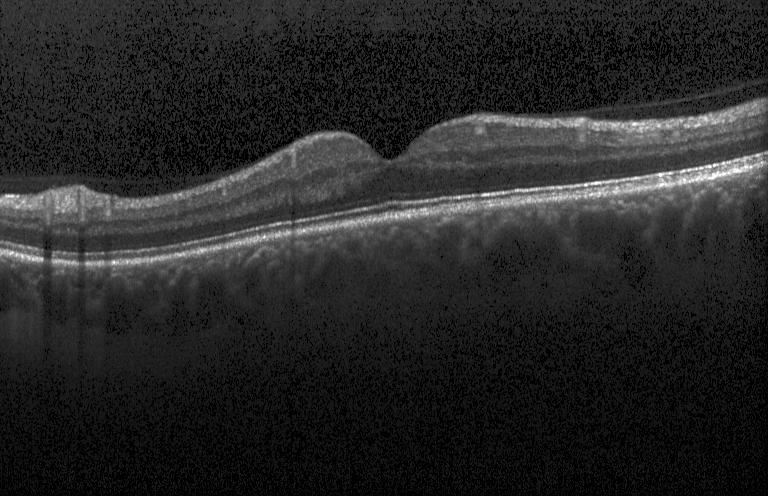
Optical coherence tomography scan · Heidelberg Spectralis.
Assessment: no evidence of CNV, DME, or drusen.